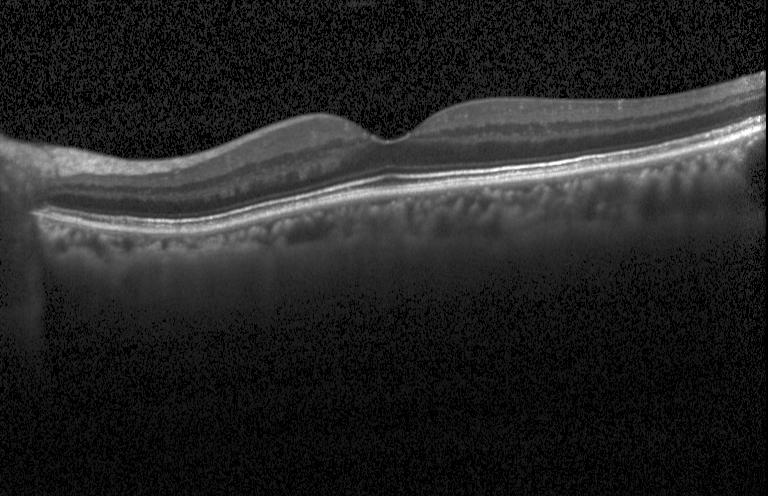

Spectral-domain optical coherence tomography, retinal OCT cross-section, instrument: Heidelberg Spectralis
Diagnosis: no choroidal neovascularization, diabetic macular edema, or drusen.